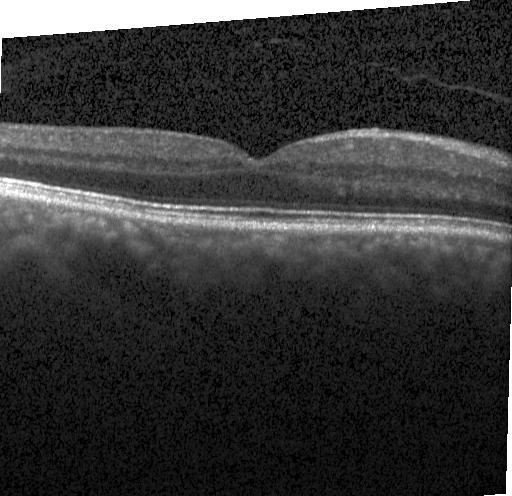
Acquired on a Heidelberg Spectralis · OCT line scan. Neither choroidal neovascularization, diabetic macular edema, nor drusen.